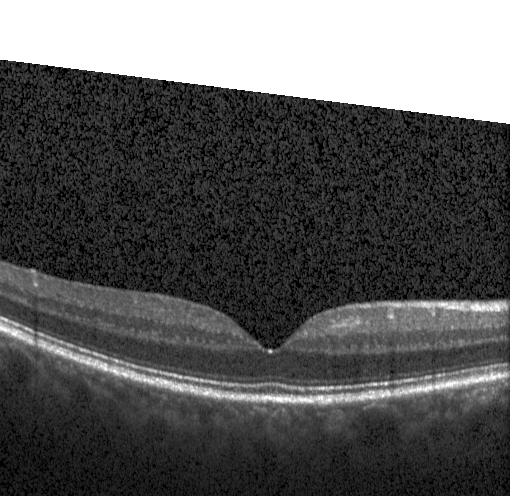 Finding: no choroidal neovascularization, no diabetic macular edema, and no drusen.